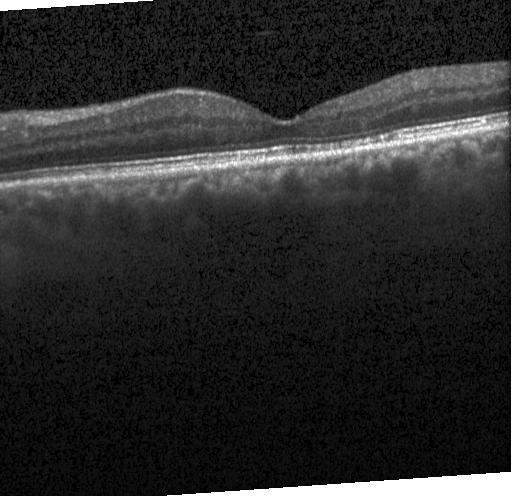
Dx: no choroidal neovascularization, diabetic macular edema, or drusen.